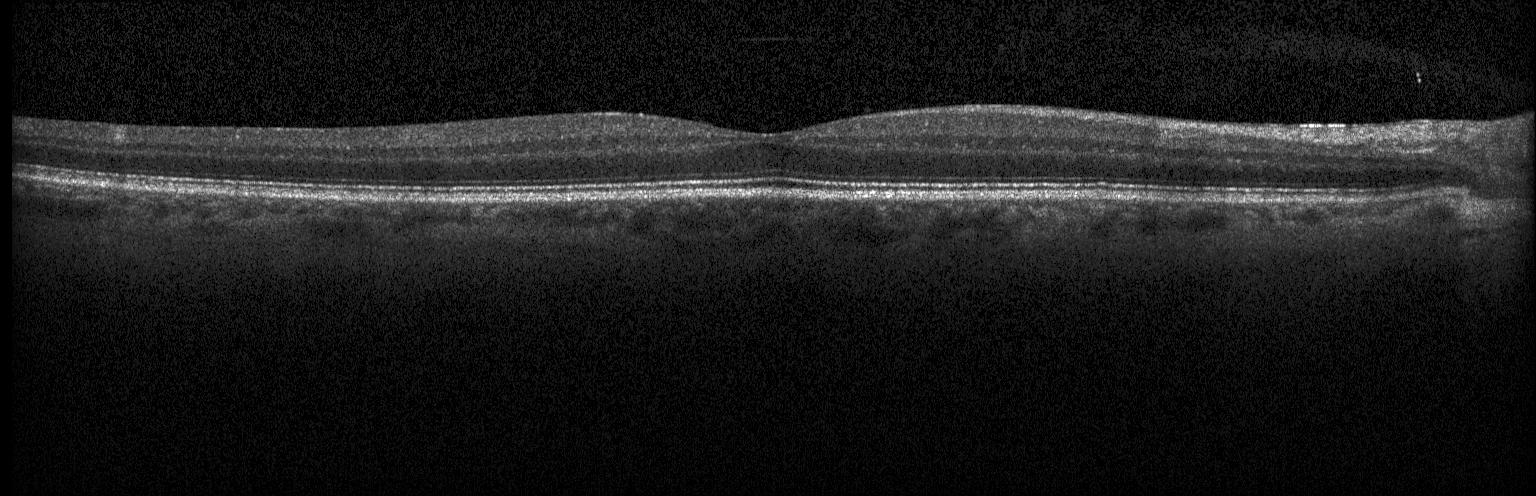
Heidelberg Spectralis · macular scan · optical coherence tomography B-scan · spectral-domain optical coherence tomography
Assessment: no choroidal neovascularization, diabetic macular edema, or drusen.